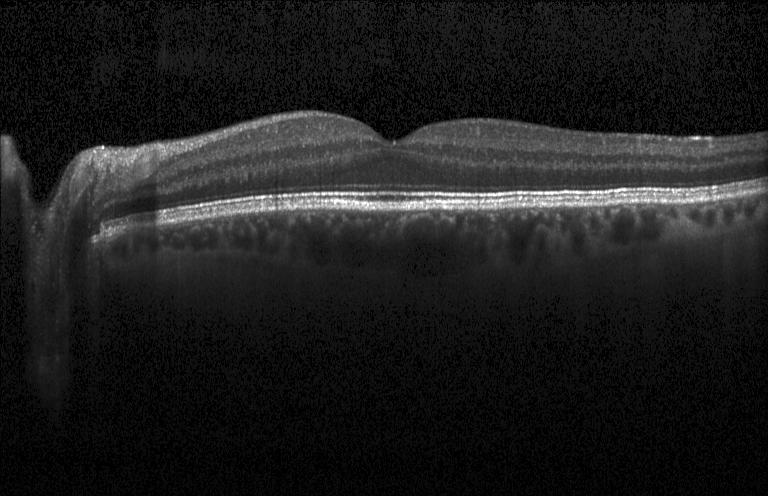

Optical coherence tomography scan.
Assessment: no evidence of choroidal neovascularization, diabetic macular edema, or drusen.